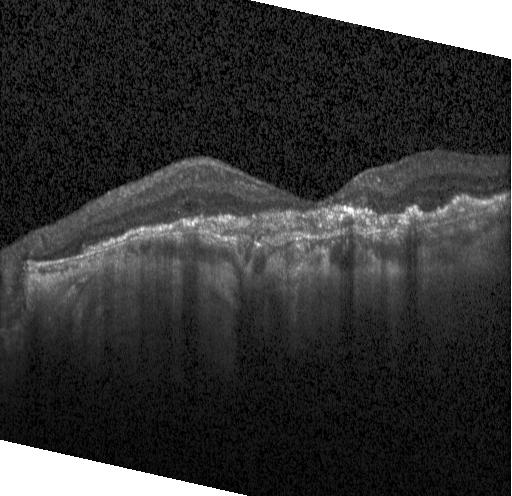
Retinal OCT cross-section showing a choroidal neovascular membrane.